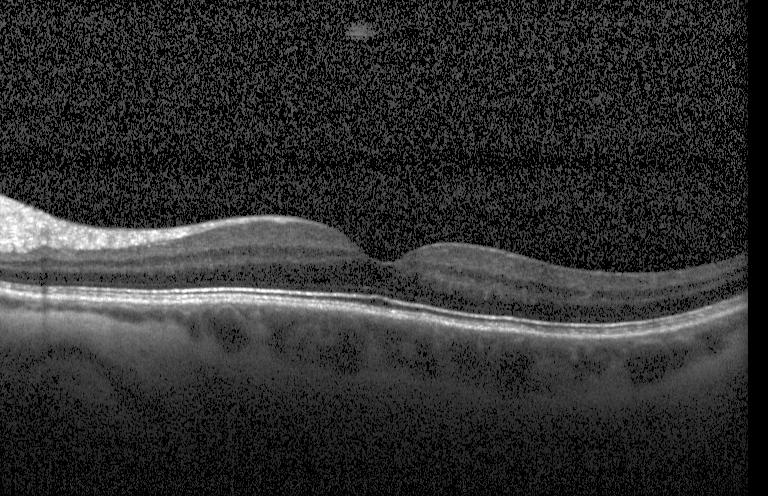 Finding: no CNV, DME, or drusen.